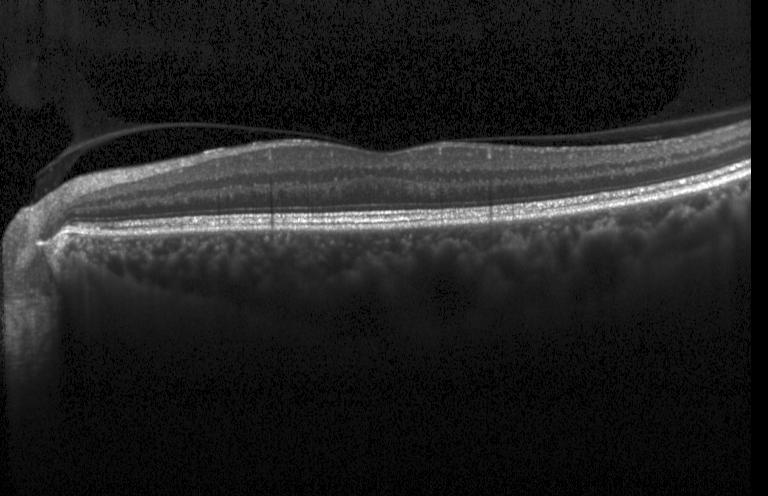
Centered on the fovea · optical coherence tomography scan · spectral-domain optical coherence tomography. Finding: no evidence of choroidal neovascularization, diabetic macular edema, or drusen.